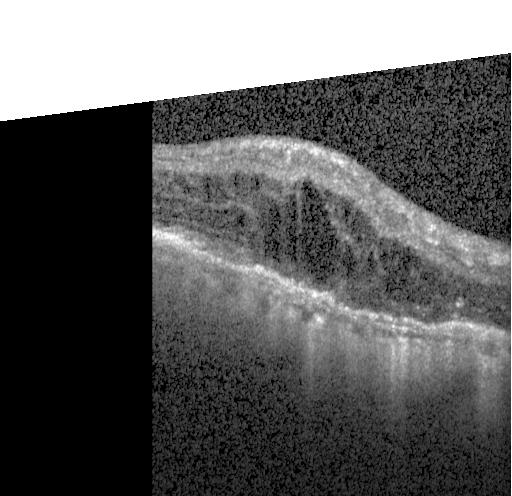

Through the macula; spectral-domain OCT; optical coherence tomography scan; Heidelberg Spectralis — Finding: a choroidal neovascular membrane.